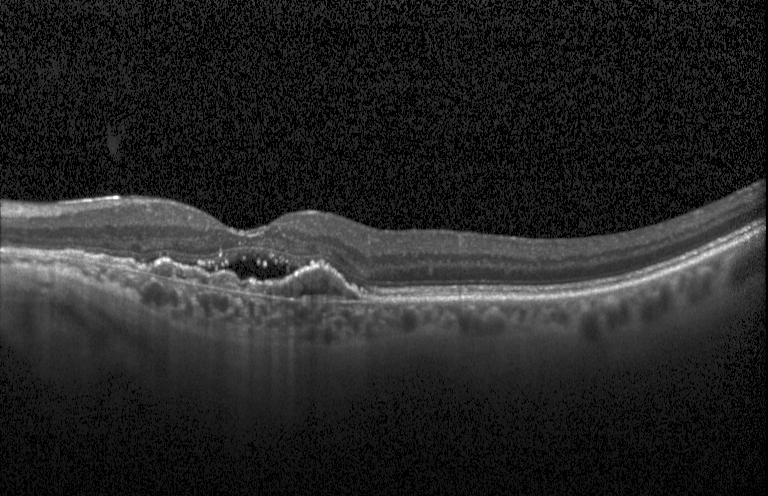

Optical coherence tomography scan — Impression: a choroidal neovascular membrane.